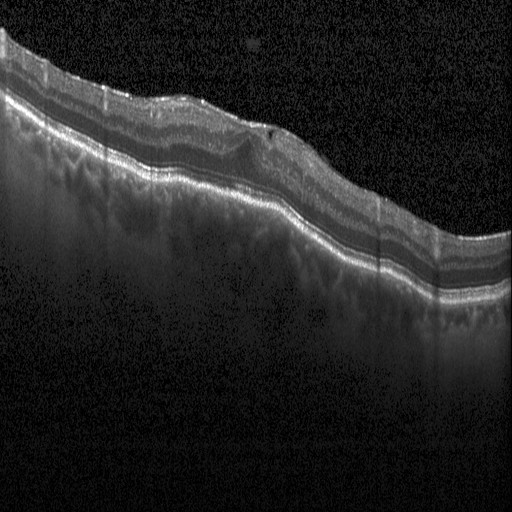
Retinal OCT B-scan
Dx: diabetic macular edema (DME).